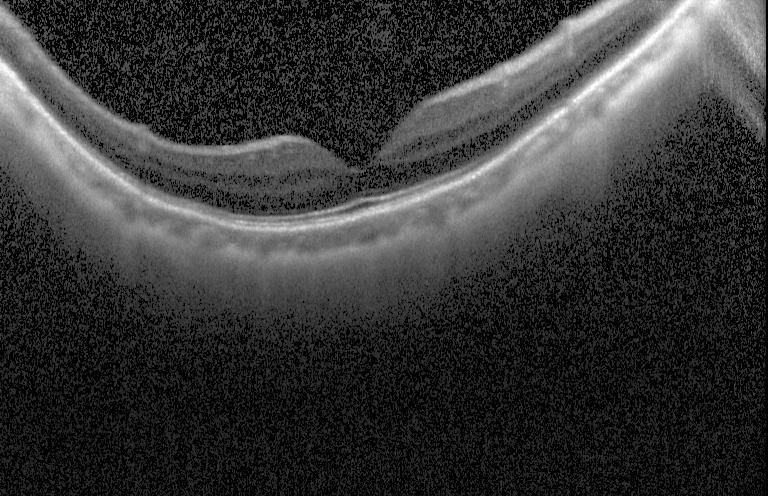
Centered on the fovea. SD-OCT. Instrument: Heidelberg Spectralis. OCT B-scan. OCT finding: no CNV, DME, or drusen.